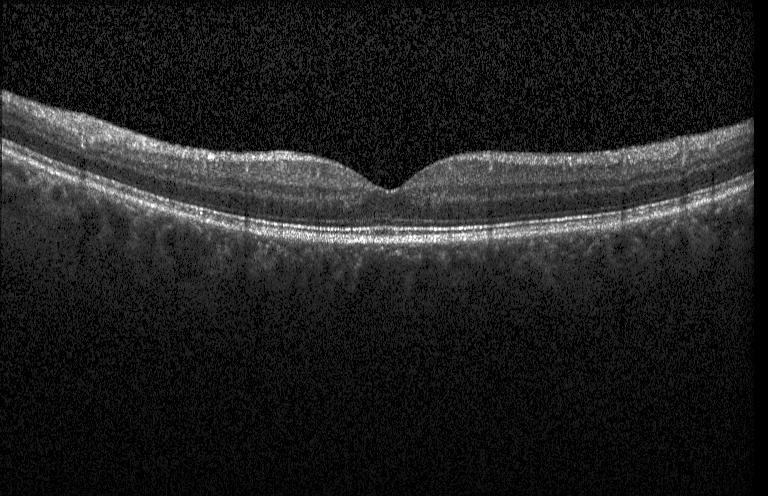 The scan shows neither CNV, DME, nor drusen.